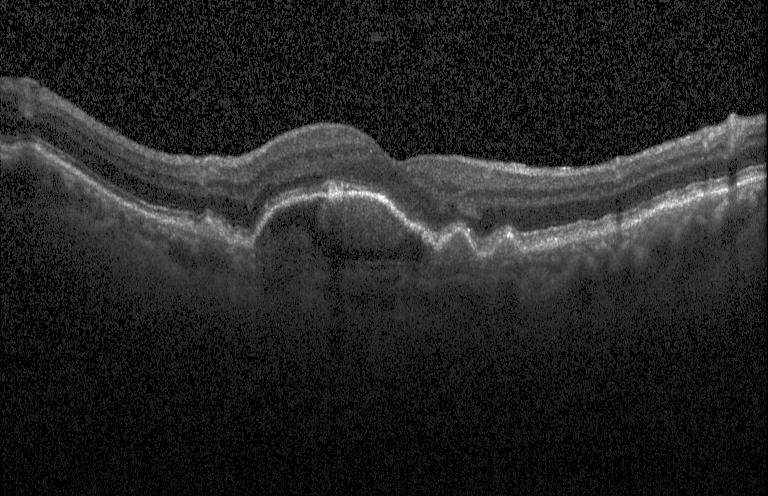
Heidelberg Spectralis OCT system, OCT line scan, spectral-domain OCT. Impression: multiple drusen.